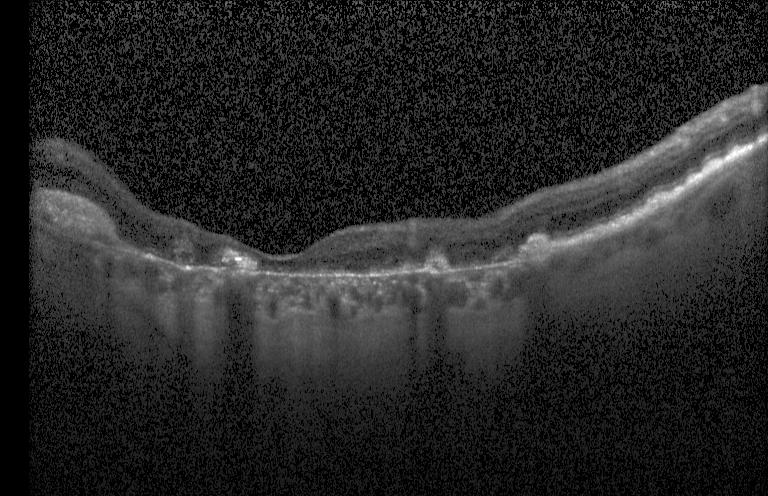 OCT B-scan; Heidelberg Spectralis. The scan shows a choroidal neovascular membrane.